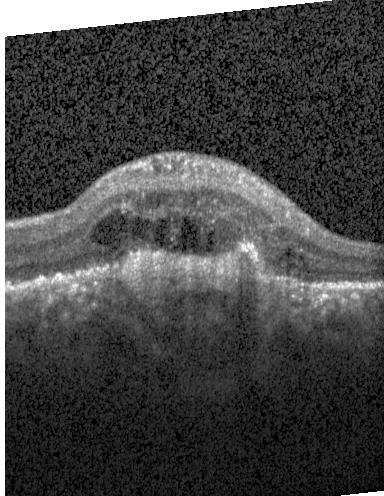
Spectral-domain optical coherence tomography · optical coherence tomography B-scan · horizontal scan through the fovea · Heidelberg Spectralis OCT system
OCT finding: CNV.